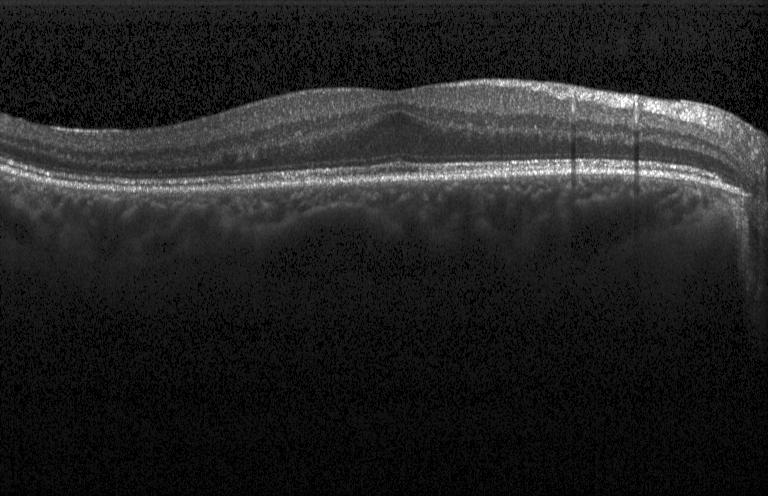 Dx: no choroidal neovascularization, no diabetic macular edema, and no drusen.